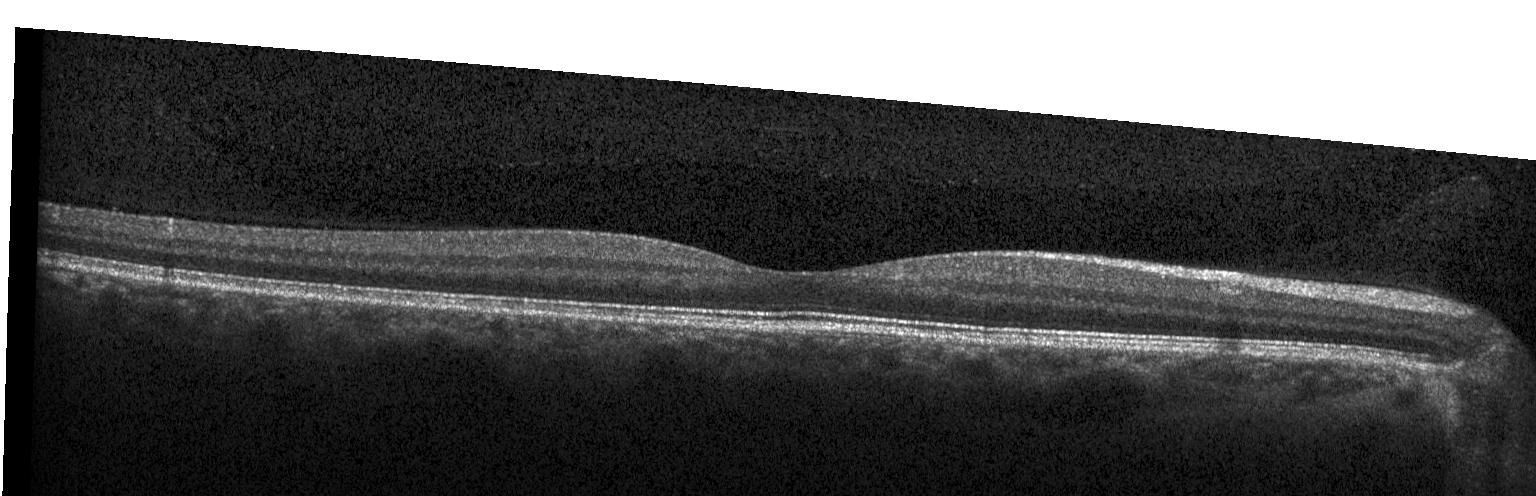
Retinal OCT B-scan, SD-OCT, horizontal scan through the fovea.
Diagnosis: neither CNV, DME, nor drusen.